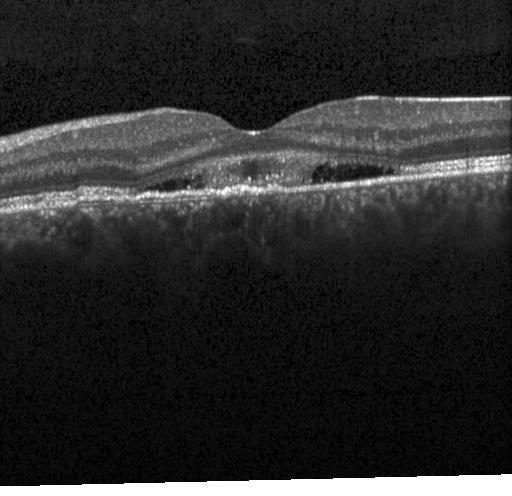 Diagnosis: CNV.